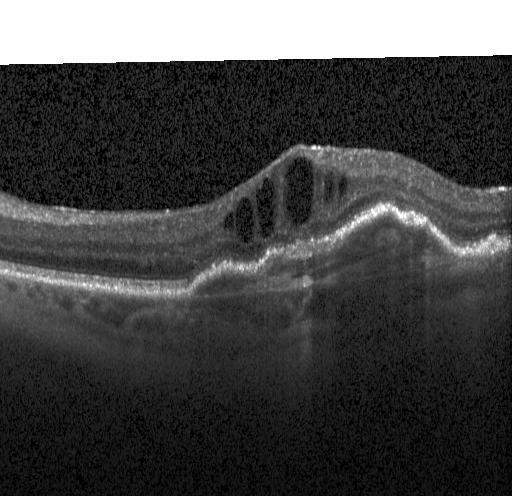
Fovea-centered; optical coherence tomography B-scan; spectral-domain optical coherence tomography; instrument: Heidelberg Spectralis — Impression: choroidal neovascularization.